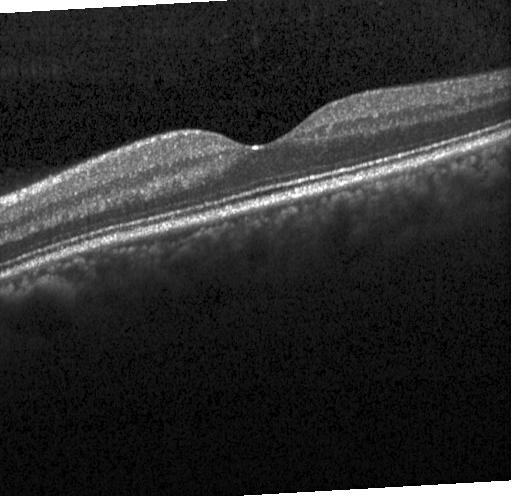 This B-scan demonstrates no choroidal neovascularization, no diabetic macular edema, and no drusen.